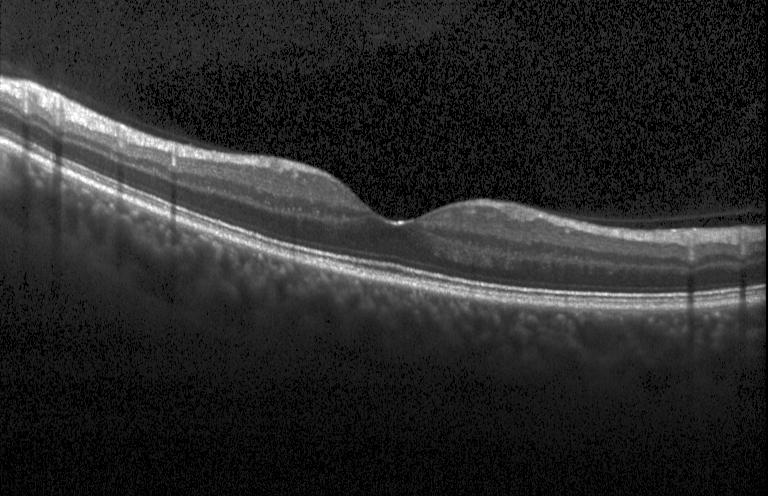 Spectral-domain OCT B-scan: no choroidal neovascularization, diabetic macular edema, or drusen.